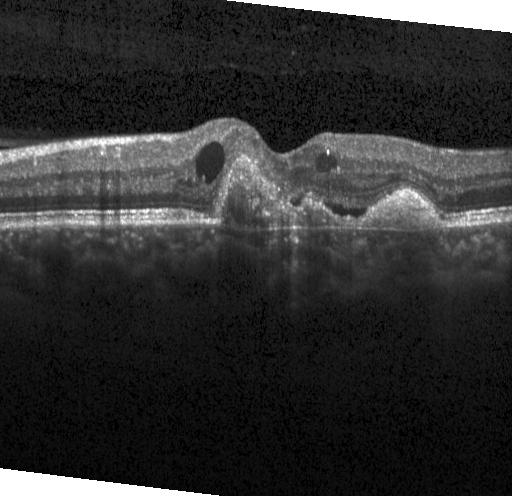
Through the macula, optical coherence tomography scan, spectral-domain optical coherence tomography
Assessment: a choroidal neovascular membrane.